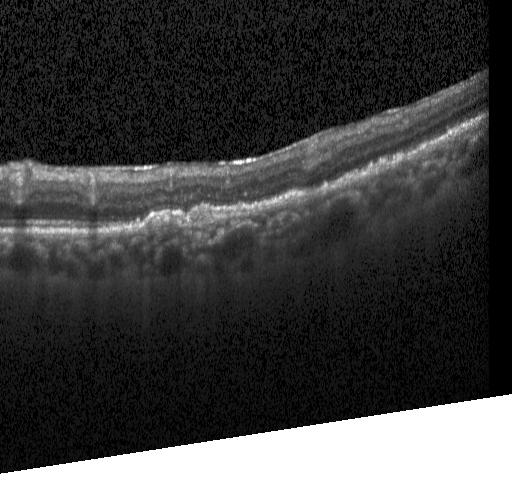
Optical coherence tomography B-scan.
Impression: CNV.